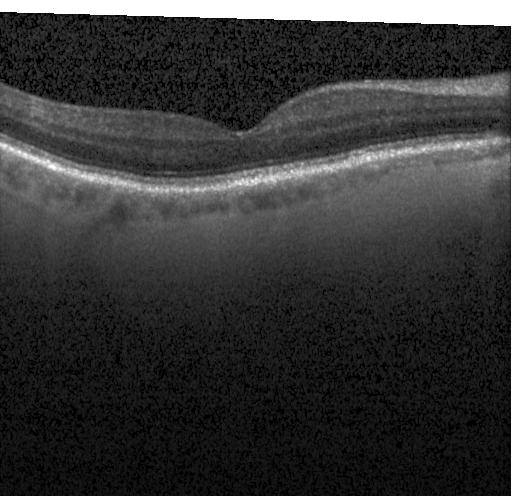

Spectral-domain OCT B-scan: neither CNV, DME, nor drusen.